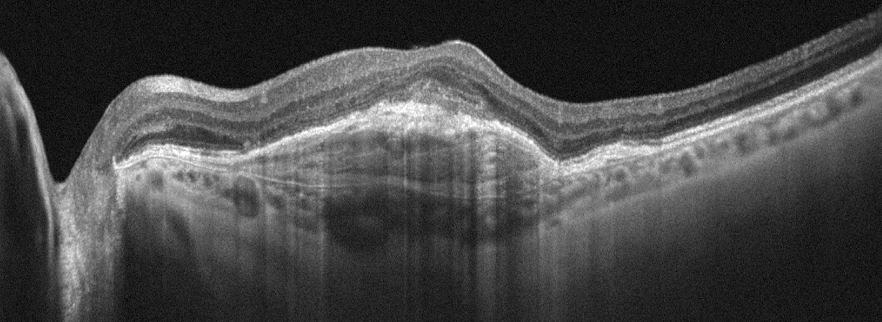

Acquired on an Optovue Avanti RTVue XR. Through the macula. Optical coherence tomography B-scan.
Age-related macular degeneration.